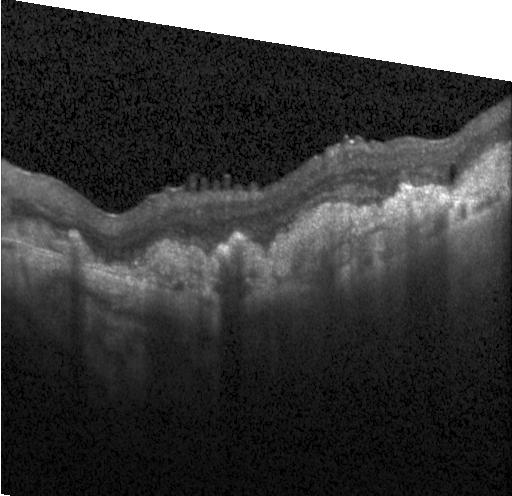

Macular OCT demonstrating a choroidal neovascular membrane.